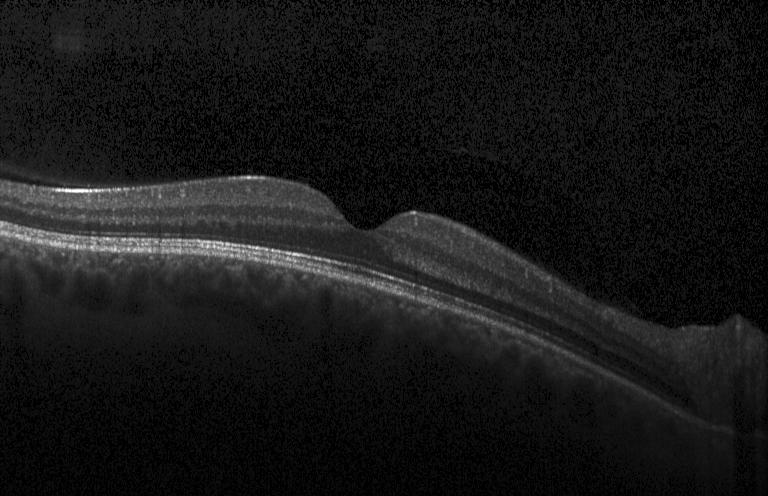

Retinal OCT B-scan. Acquired on a Heidelberg Spectralis. Diagnosis: no evidence of CNV, DME, or drusen.